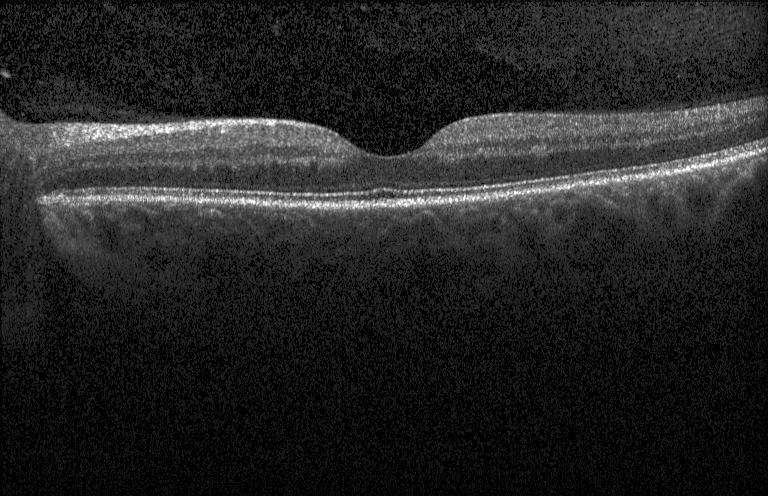
Macular scan; retinal OCT B-scan. This B-scan demonstrates no CNV, DME, or drusen.